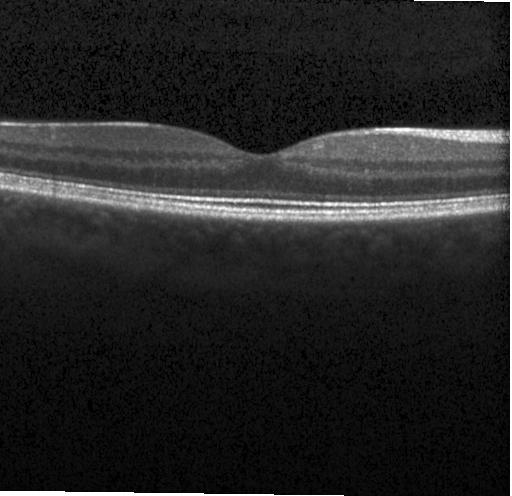
OCT B-scan showing no CNV, DME, or drusen.